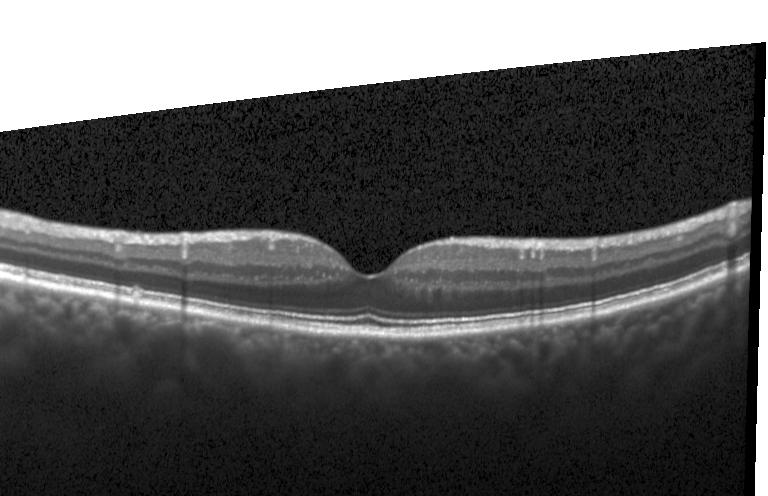 Finding: no CNV, DME, or drusen.